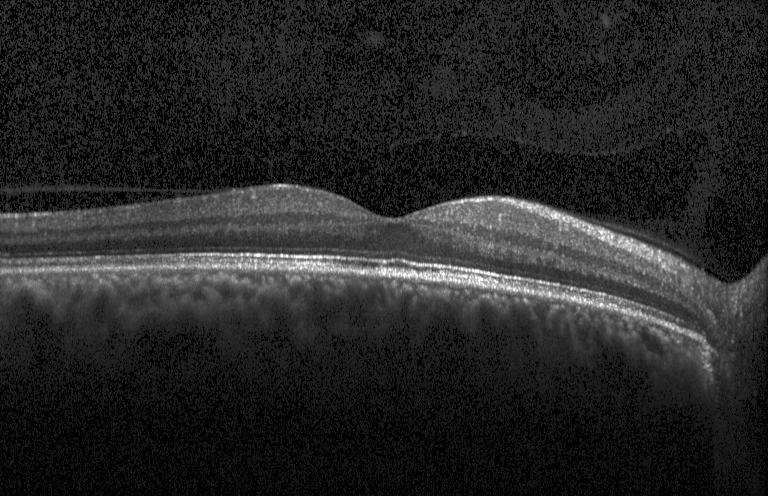

Retinal OCT cross-section
Diagnosis: neither choroidal neovascularization, diabetic macular edema, nor drusen.